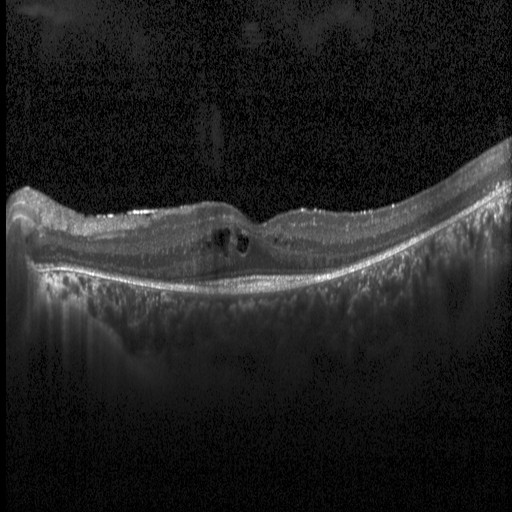 OCT B-scan.
Impression: diabetic macular edema (DME).